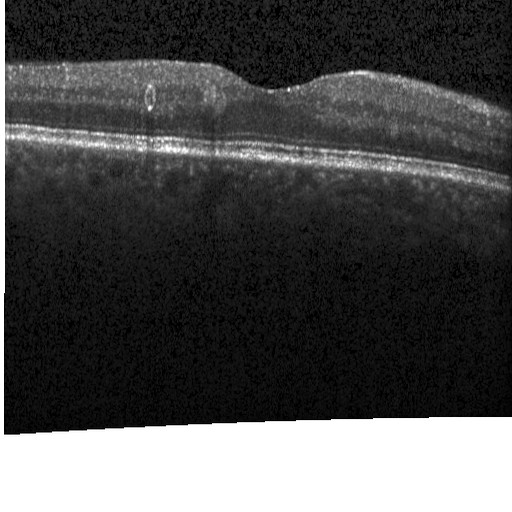
OCT B-scan. Diagnosis: DME.